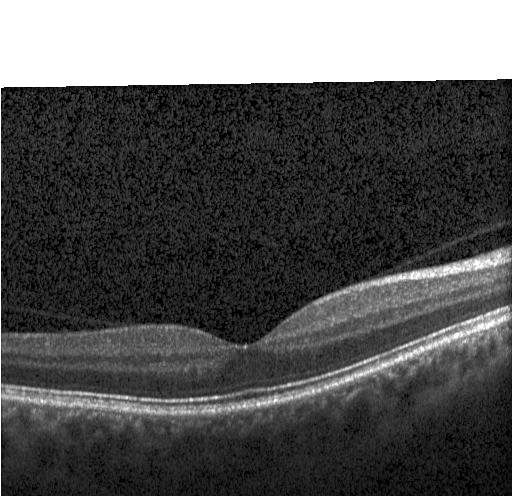

Optical coherence tomography B-scan · centered on the fovea. Impression: neither CNV, DME, nor drusen.